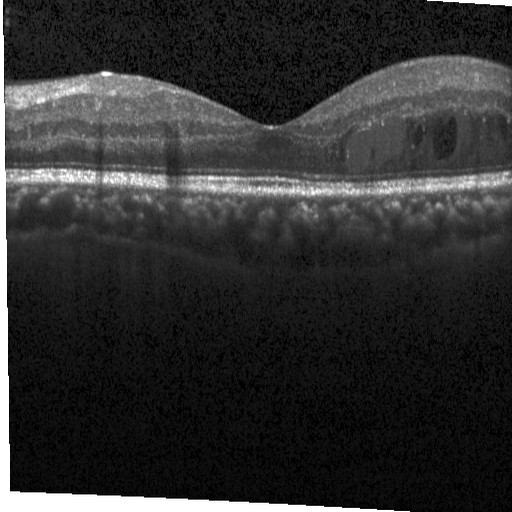
Macular scan · OCT B-scan · instrument: Heidelberg Spectralis. This B-scan demonstrates DME.